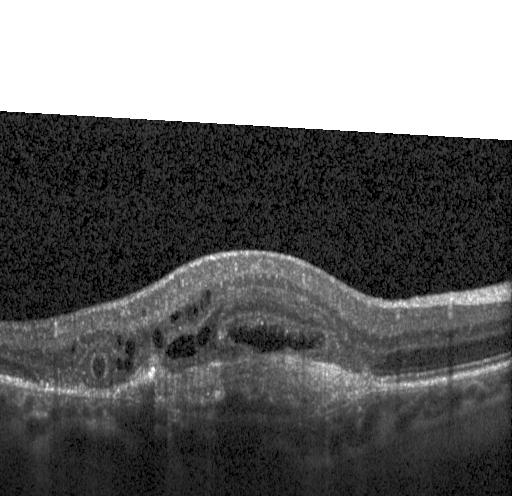
Assessment: choroidal neovascularization.